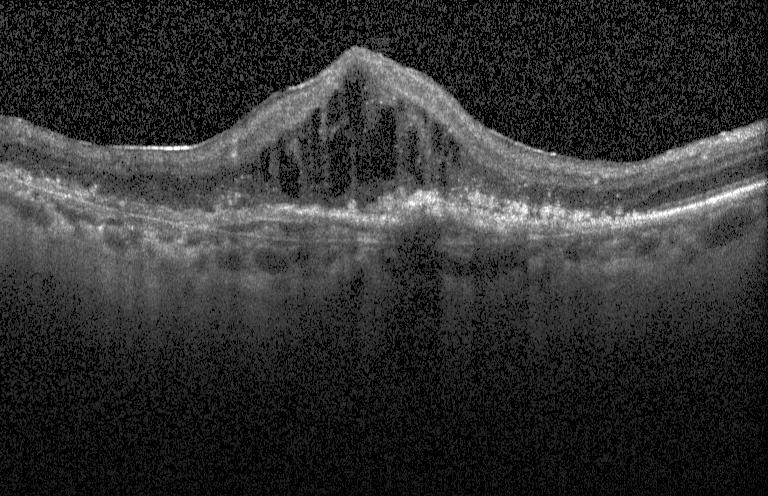

OCT scan showing choroidal neovascularization (CNV).